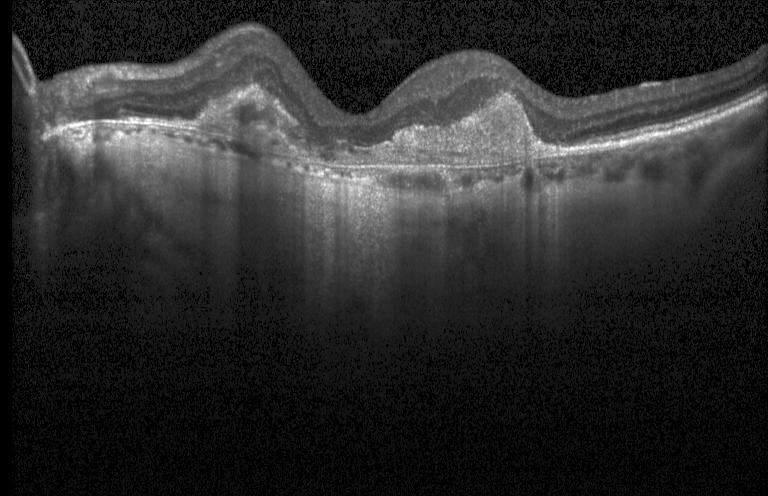 OCT B-scan. Impression: a choroidal neovascular membrane.